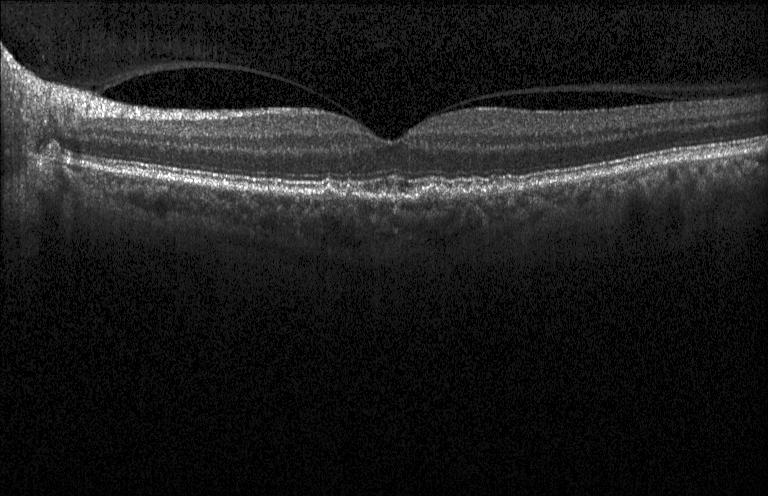
OCT finding: sub-RPE drusenoid deposits.